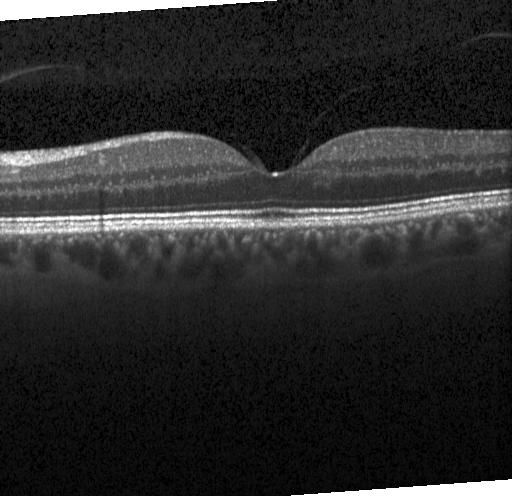

Spectral-domain OCT; horizontal scan through the fovea; retinal OCT B-scan; acquired on a Heidelberg Spectralis.
This B-scan demonstrates neither CNV, DME, nor drusen.